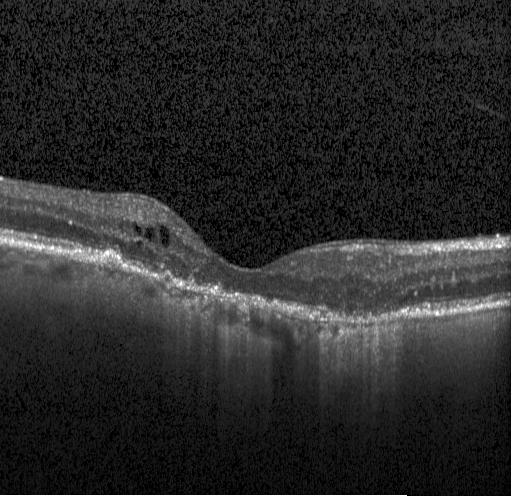
Acquired on a Heidelberg Spectralis. OCT line scan
This B-scan demonstrates a choroidal neovascular membrane.